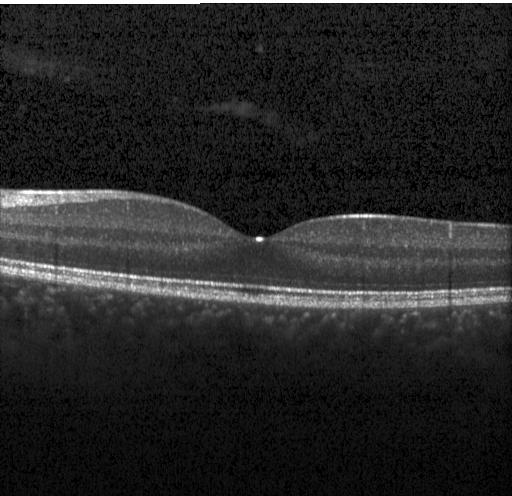 Retinal OCT B-scan. Dx: no choroidal neovascularization, diabetic macular edema, or drusen.